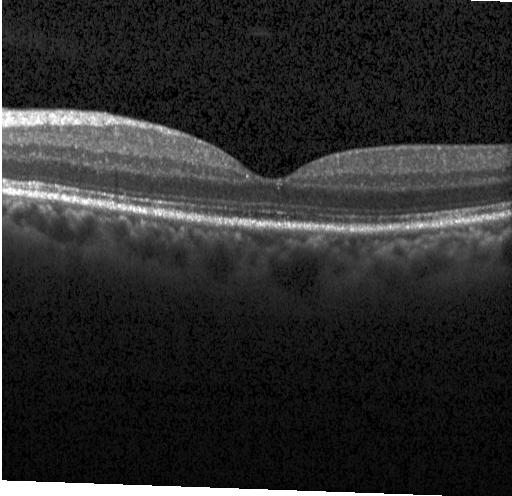
Optical coherence tomography B-scan.
Dx: no evidence of choroidal neovascularization, diabetic macular edema, or drusen.